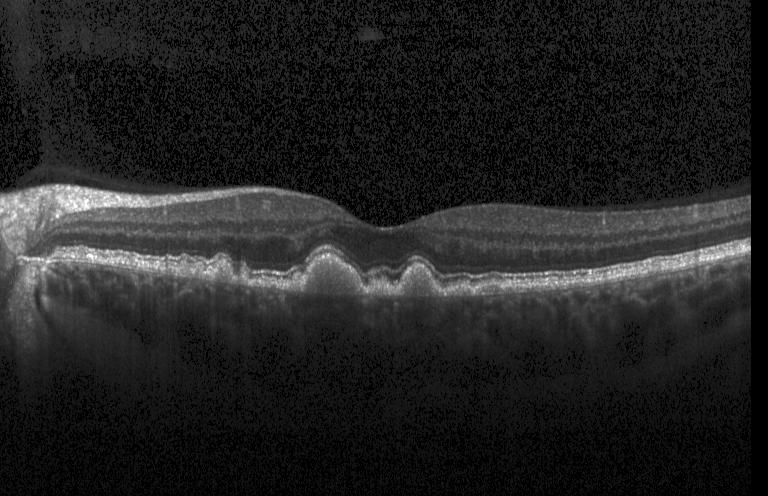

Retinal OCT cross-section; SD-OCT; centered on the fovea; Heidelberg Spectralis OCT system. Impression: drusen.